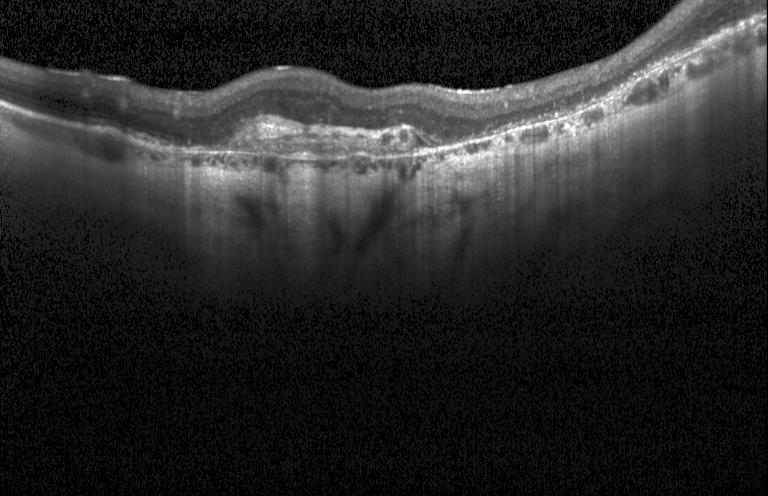

The scan shows choroidal neovascularization.